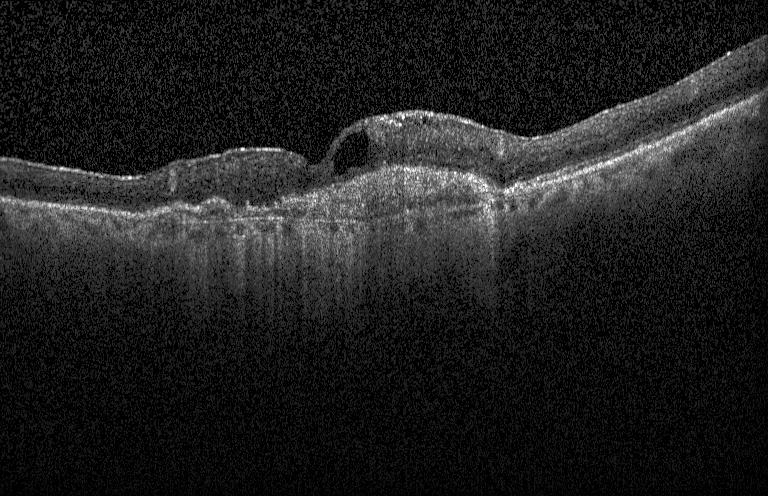
Assessment: choroidal neovascularization (CNV).